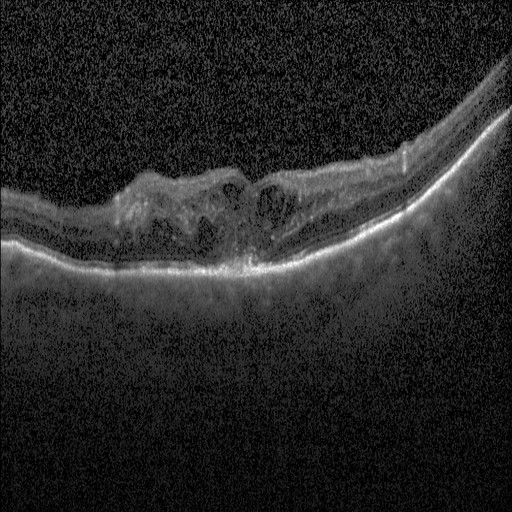

Spectral-domain optical coherence tomography. Acquired on a Heidelberg Spectralis. Retinal OCT cross-section. Diabetic macular edema (DME).